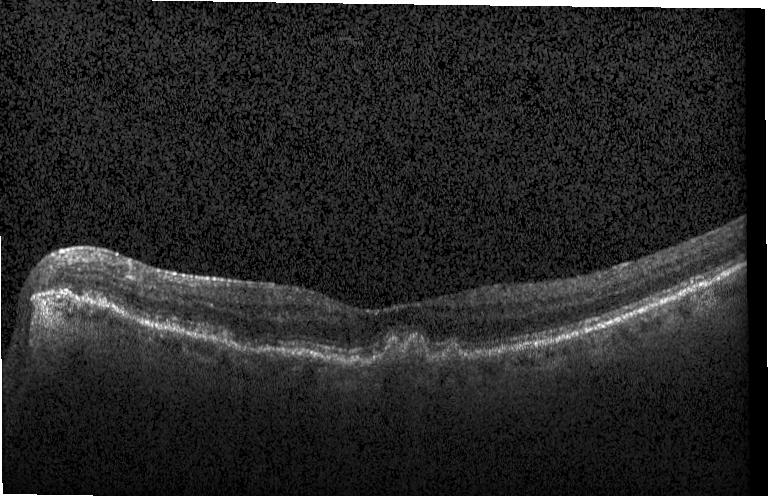 Spectral-domain optical coherence tomography · Heidelberg Spectralis OCT system · OCT B-scan · fovea-centered.
Dx: sub-RPE drusenoid deposits.